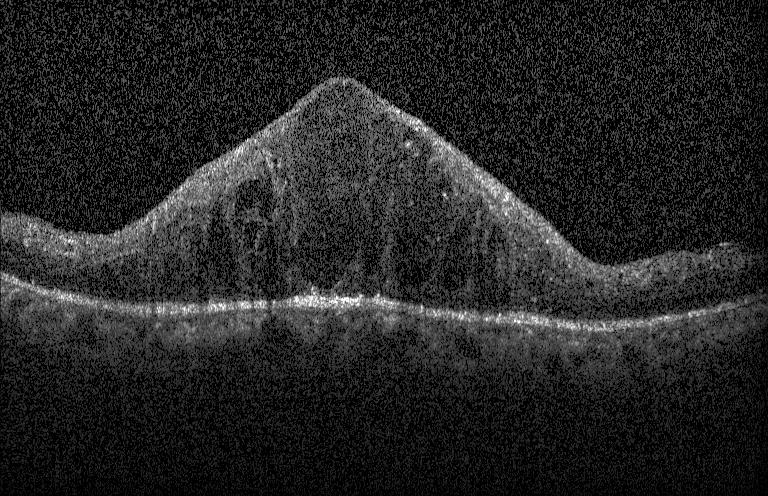

OCT line scan, through the macula, Heidelberg Spectralis, spectral-domain optical coherence tomography.
Assessment: diabetic macular edema (DME).